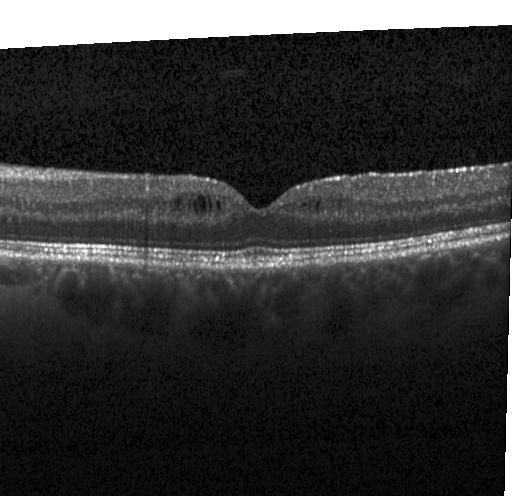
Optical coherence tomography scan. Spectral-domain OCT. Heidelberg Spectralis. Through the macula. OCT finding: DME.